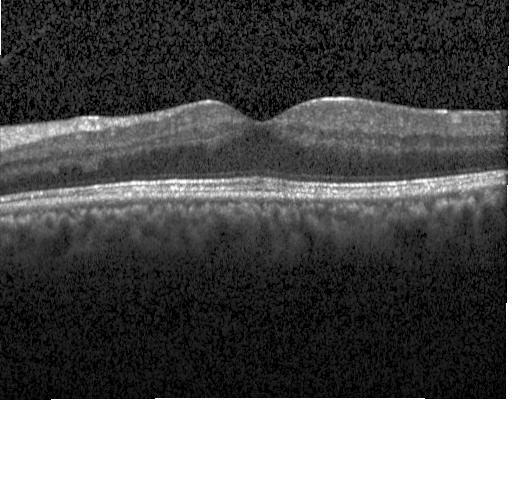

SD-OCT, retinal OCT cross-section, centered on the fovea
No choroidal neovascularization, no diabetic macular edema, and no drusen.